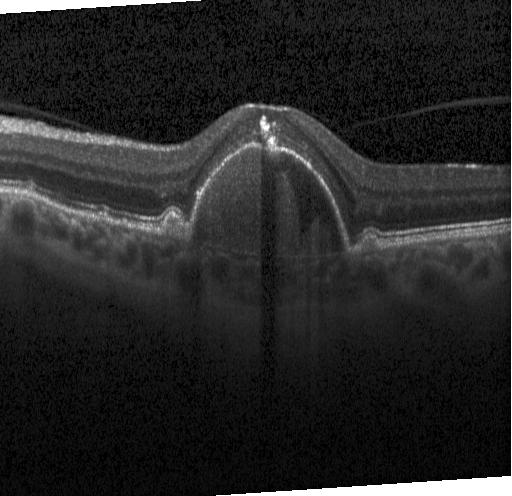 Retinal OCT B-scan, through the macula. The scan shows choroidal neovascularization (CNV).